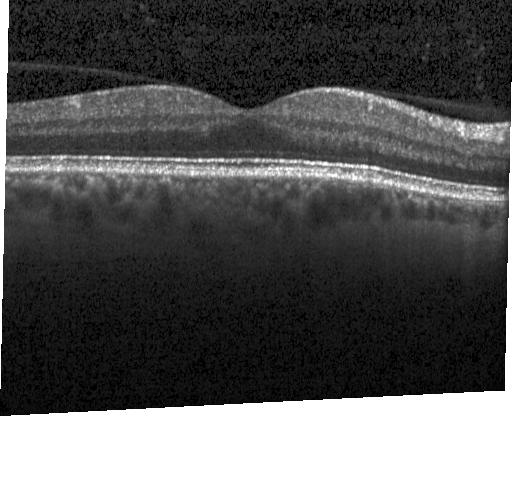
Optical coherence tomography B-scan. Fovea-centered. Spectral-domain optical coherence tomography. Finding: no CNV, no DME, and no drusen.